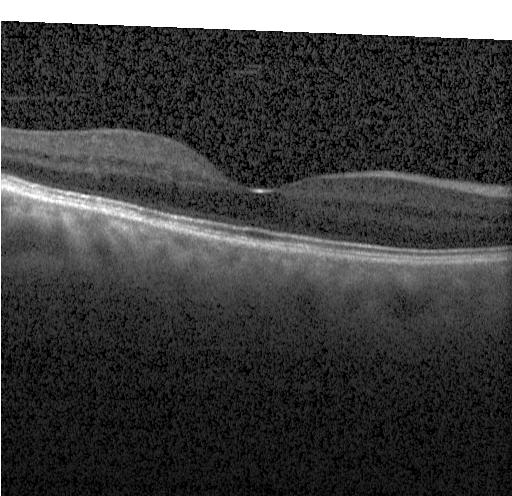

OCT line scan. Instrument: Heidelberg Spectralis. Spectral-domain optical coherence tomography — Neither choroidal neovascularization, diabetic macular edema, nor drusen.